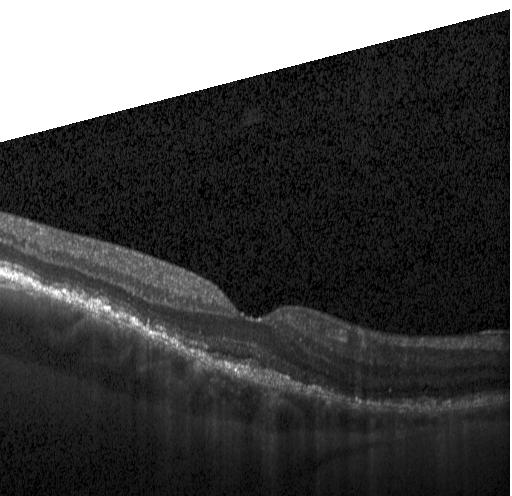
Spectral-domain OCT B-scan: choroidal neovascularization.